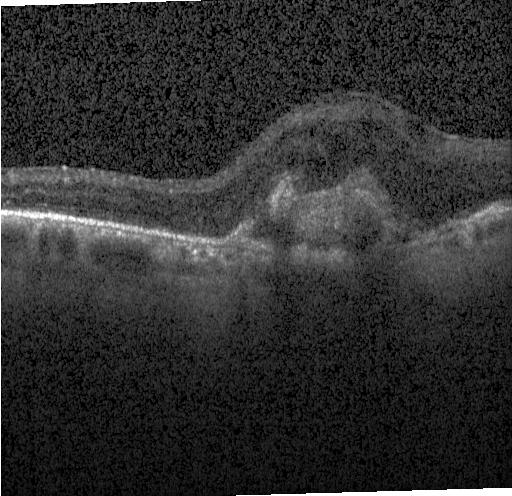
Spectral-domain optical coherence tomography · Heidelberg Spectralis · macular scan · retinal OCT B-scan. Finding: CNV.